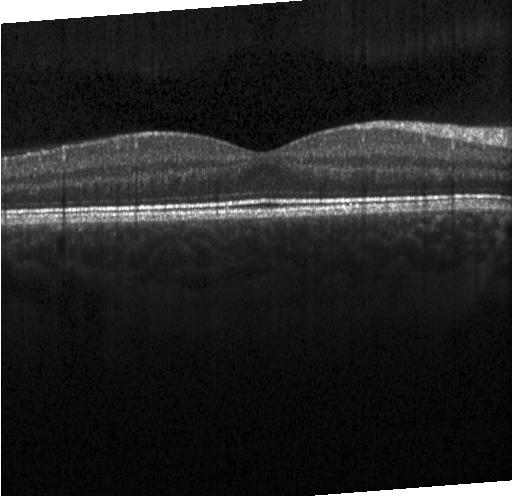
Centered on the fovea, SD-OCT, retinal OCT B-scan, Heidelberg Spectralis OCT system — Impression: no evidence of choroidal neovascularization, diabetic macular edema, or drusen.